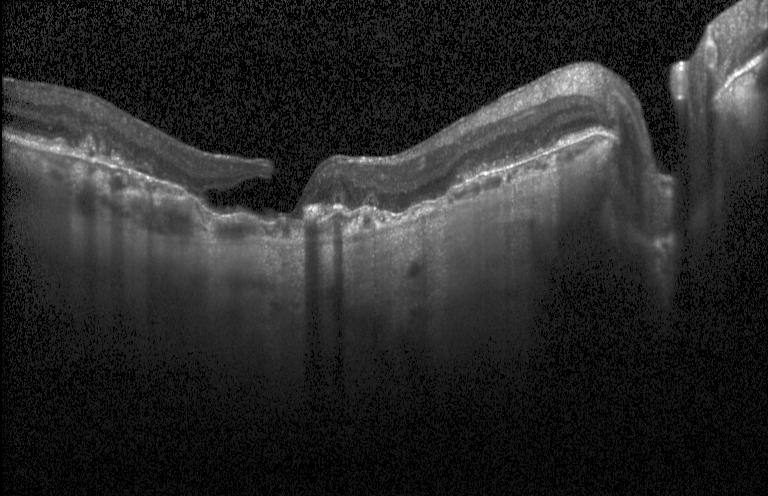 Fovea-centered. Spectral-domain optical coherence tomography. Retinal OCT cross-section. Heidelberg Spectralis — OCT finding: a choroidal neovascular membrane.